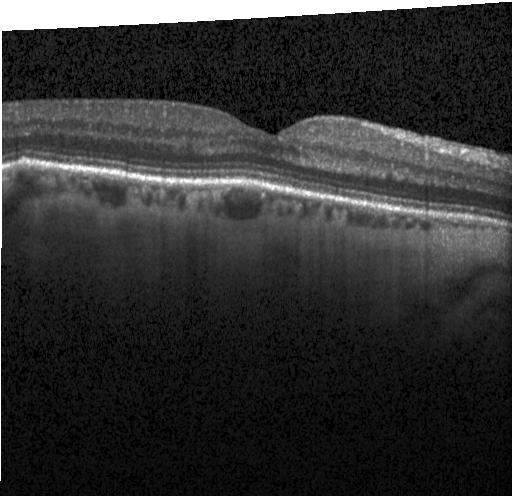 OCT scan showing no choroidal neovascularization, diabetic macular edema, or drusen.